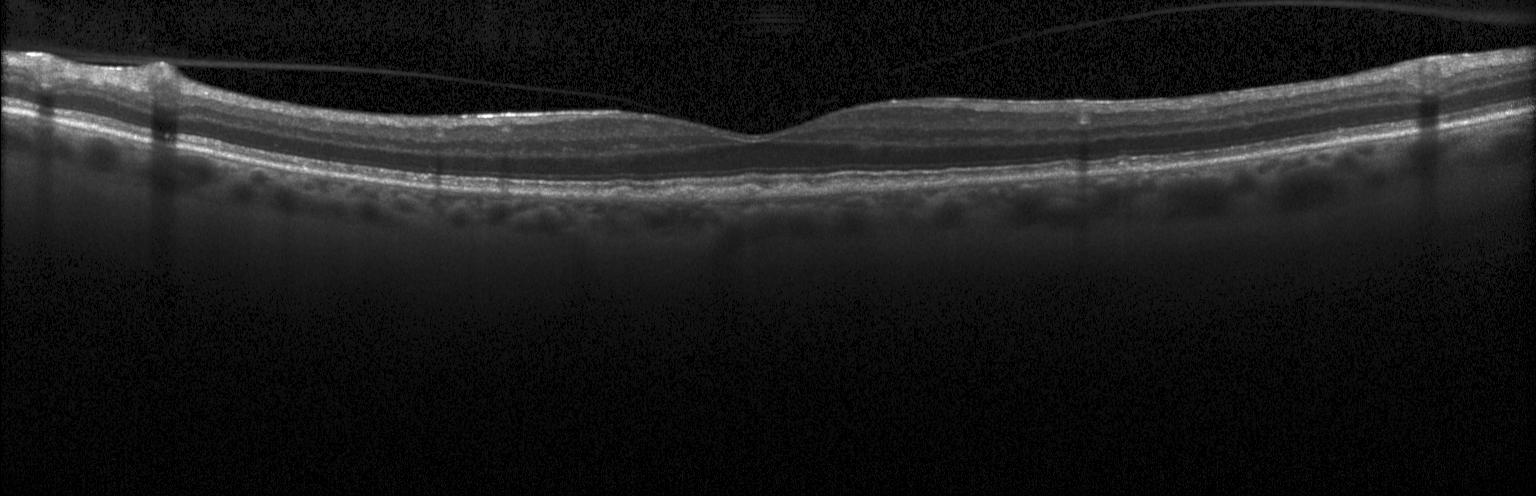 The scan shows drusen.